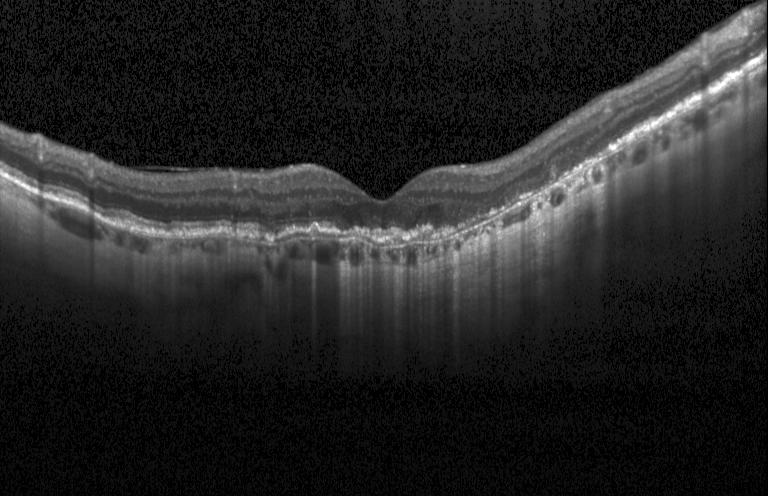

Retinal OCT cross-section showing a choroidal neovascular membrane.